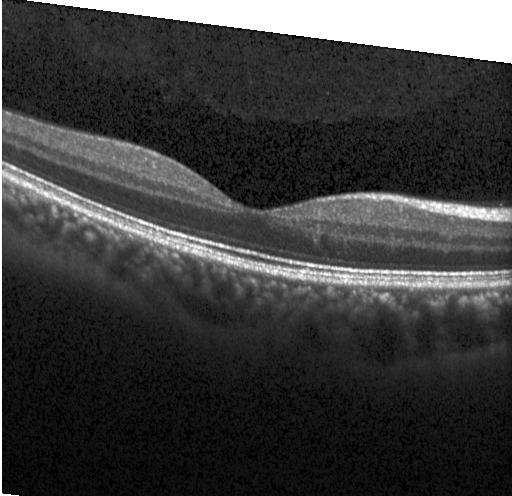 Heidelberg Spectralis OCT system. Retinal OCT B-scan. Through the macula.
Impression: no evidence of CNV, DME, or drusen.